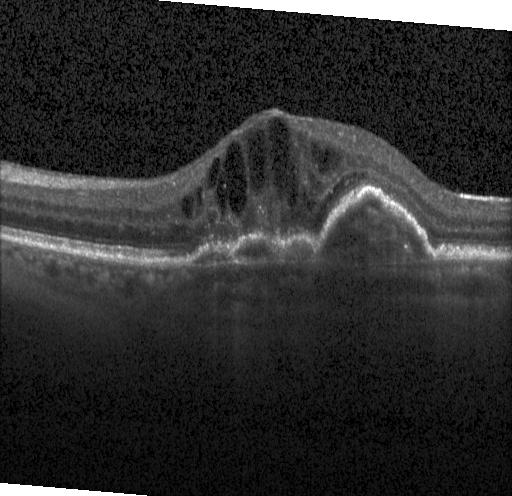

Spectral-domain optical coherence tomography; OCT B-scan.
Diagnosis: choroidal neovascularization.